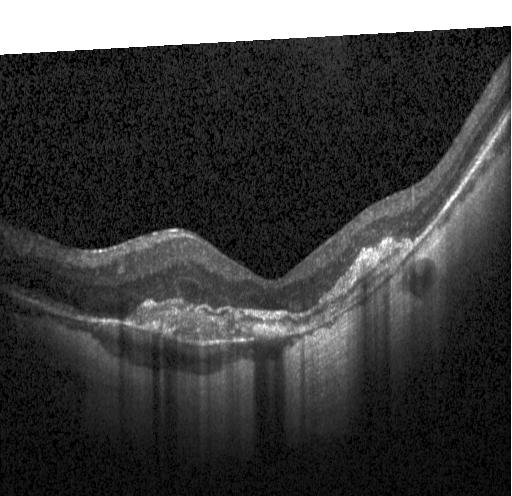

Diagnosis: choroidal neovascularization.